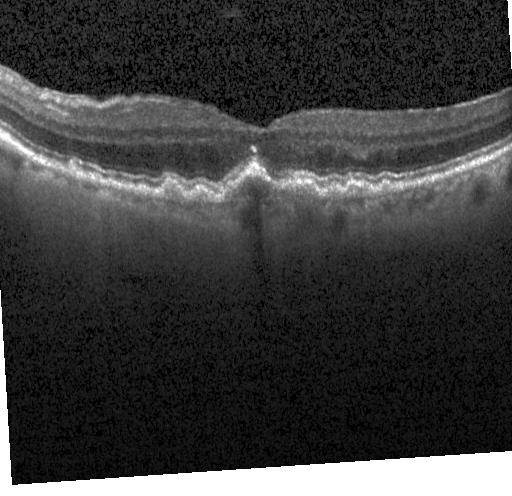 Spectral-domain optical coherence tomography, optical coherence tomography B-scan, instrument: Heidelberg Spectralis — Macular OCT: a choroidal neovascular membrane.